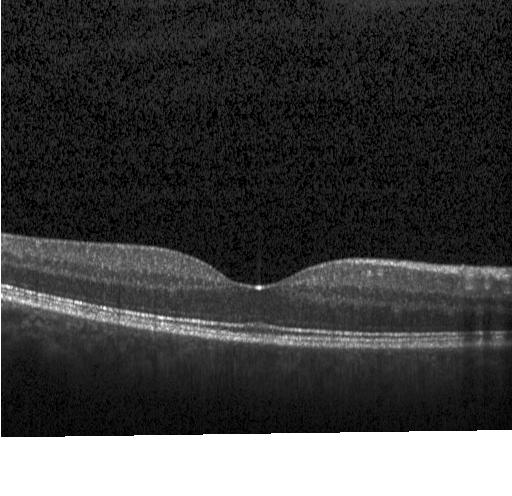
Dx: no choroidal neovascularization, diabetic macular edema, or drusen.